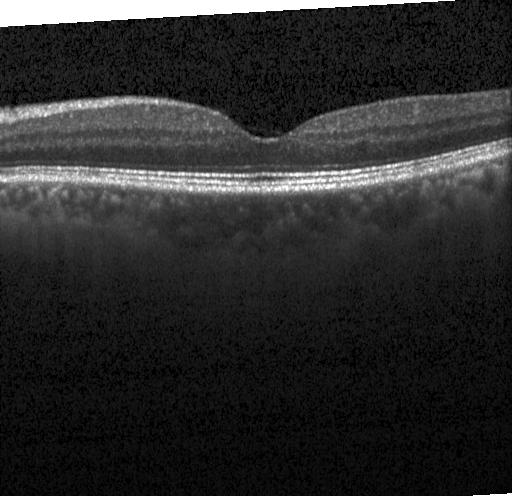
Finding: neither CNV, DME, nor drusen.